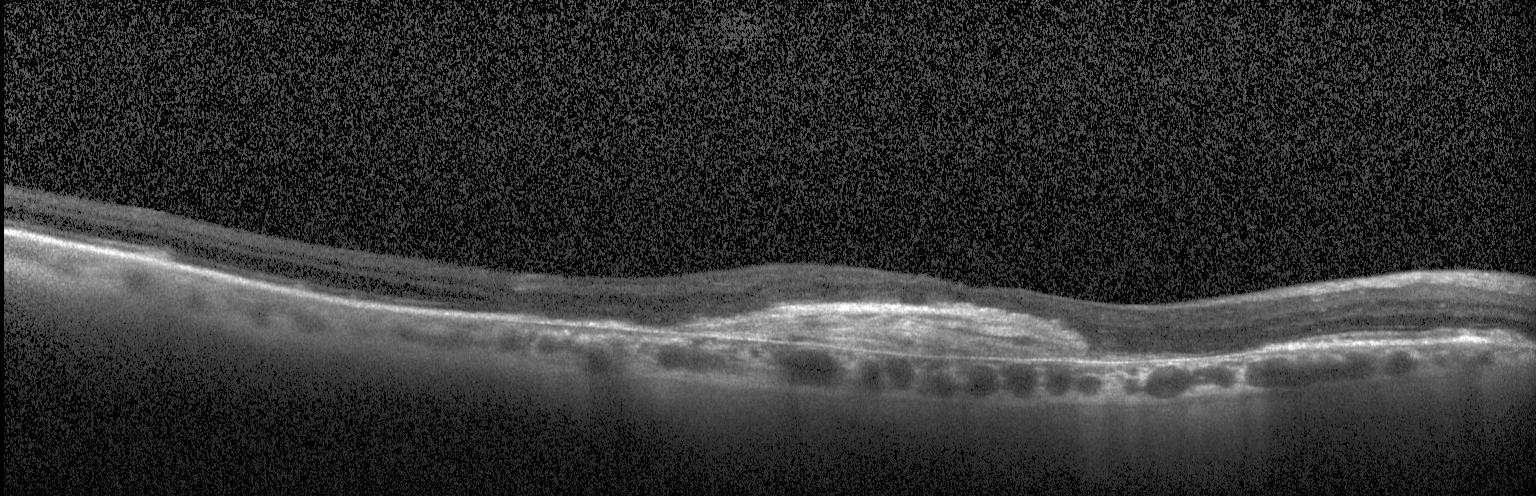
Fovea-centered. Retinal OCT cross-section. SD-OCT. Instrument: Heidelberg Spectralis. Finding: choroidal neovascularization (CNV).